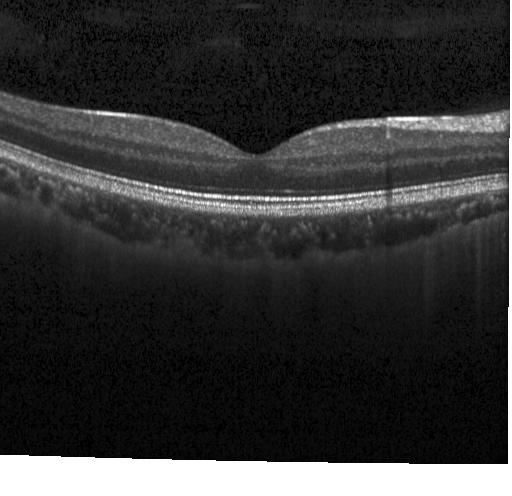 OCT finding: no evidence of choroidal neovascularization, diabetic macular edema, or drusen.